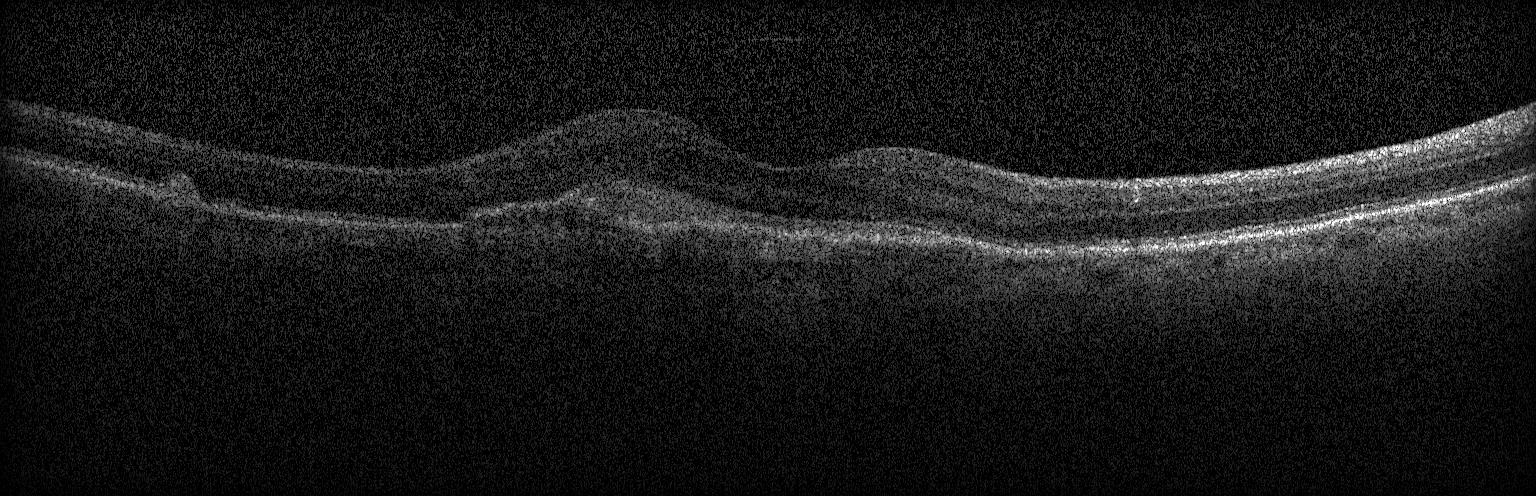
Heidelberg Spectralis, spectral-domain optical coherence tomography, retinal OCT cross-section, macular scan — Macular OCT: a choroidal neovascular membrane.